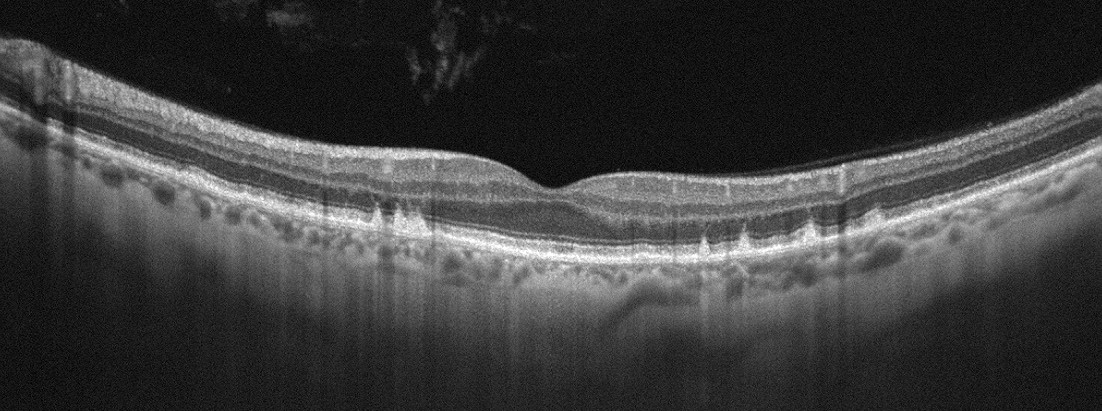

OCT B-scan — Assessment: age-related macular degeneration.